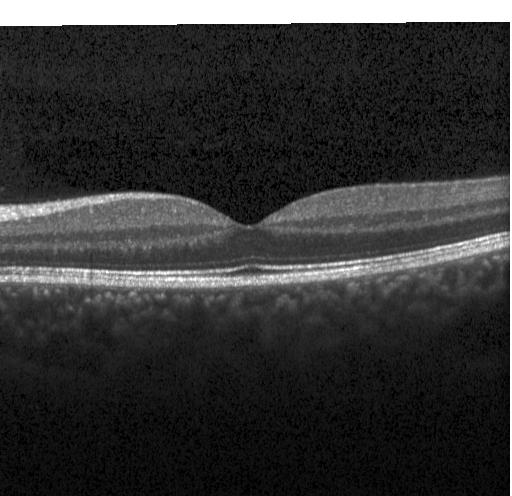
Retinal OCT cross-section showing no choroidal neovascularization, no diabetic macular edema, and no drusen.